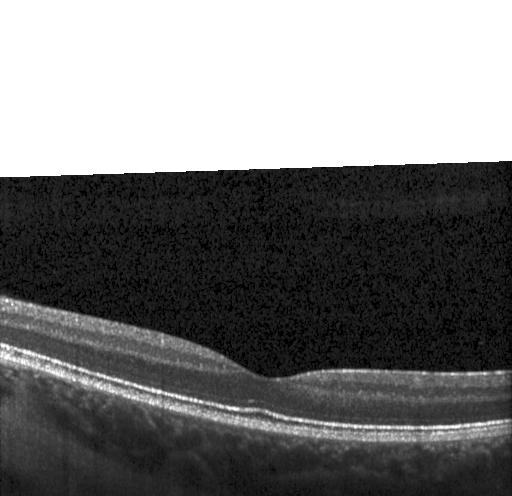
Finding: no choroidal neovascularization, no diabetic macular edema, and no drusen.